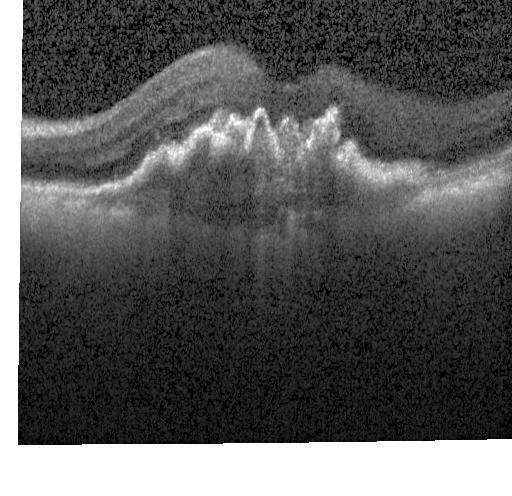 Optical coherence tomography B-scan, SD-OCT.
Diagnosis: choroidal neovascularization.